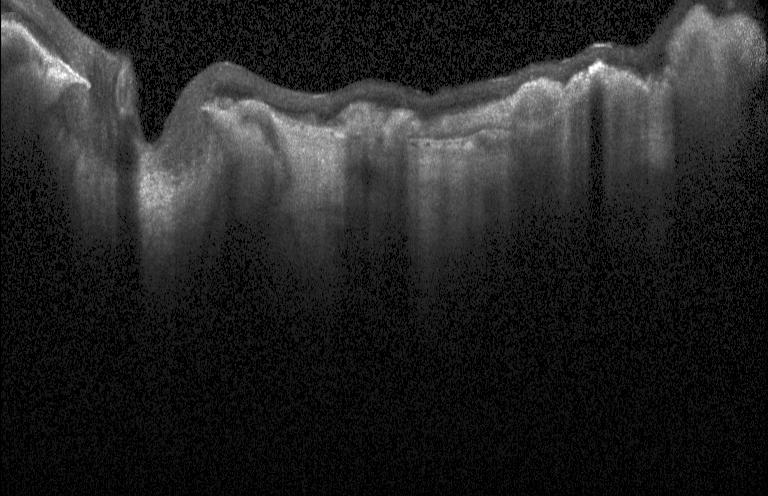

Retinal OCT cross-section, instrument: Heidelberg Spectralis. Diagnosis: choroidal neovascularization.